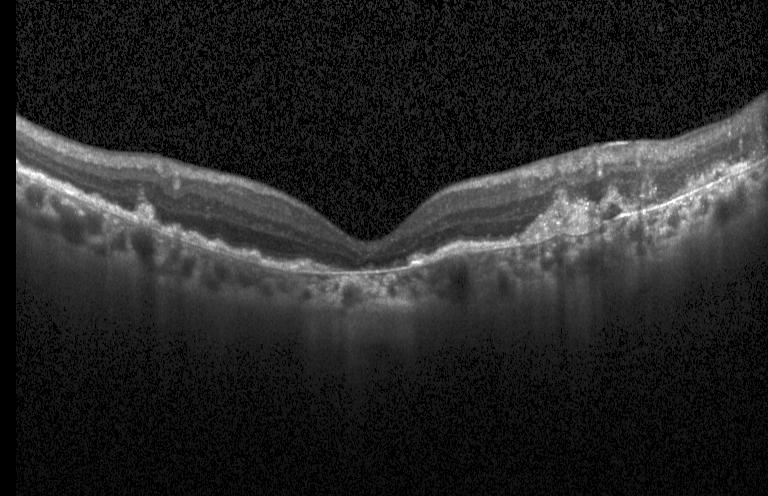 Retinal OCT cross-section, spectral-domain optical coherence tomography — Finding: a choroidal neovascular membrane.